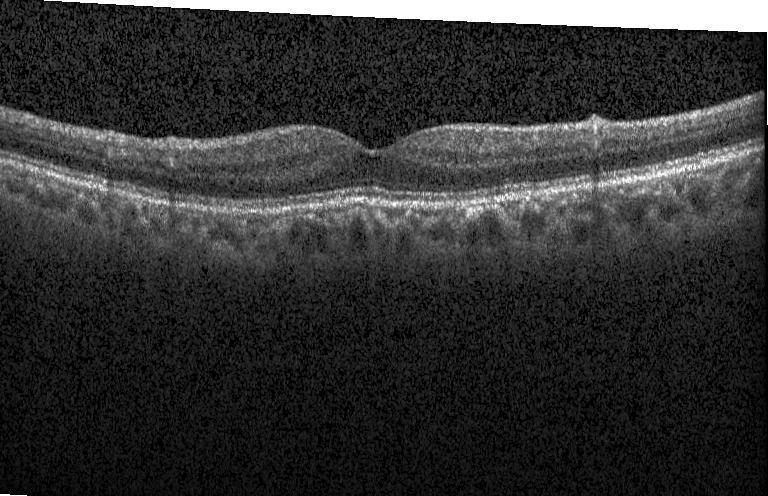
Macular OCT demonstrating neither CNV, DME, nor drusen.